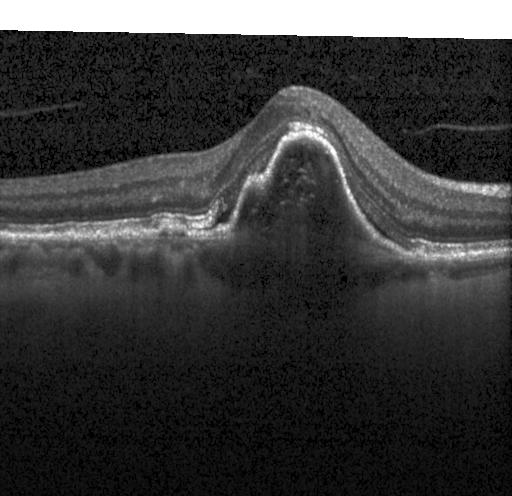 The scan shows CNV.